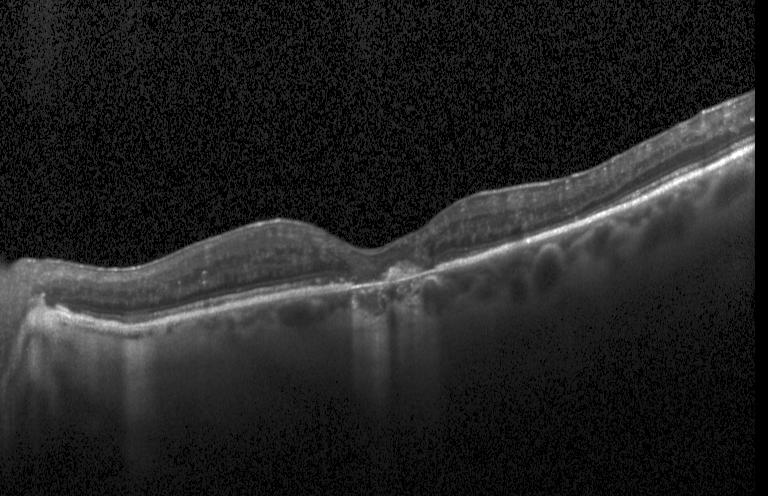 A choroidal neovascular membrane.